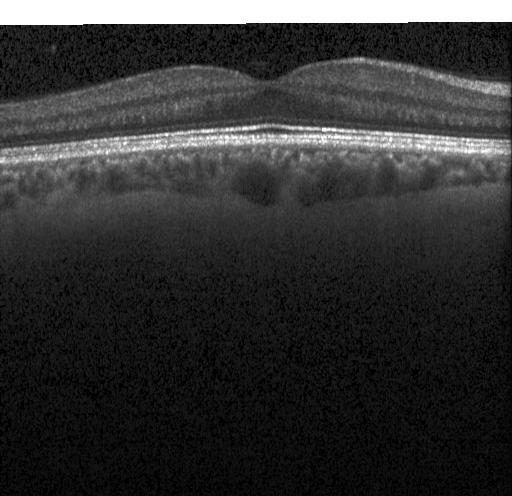

Instrument: Heidelberg Spectralis, spectral-domain optical coherence tomography, fovea-centered, optical coherence tomography scan.
The scan shows no choroidal neovascularization, no diabetic macular edema, and no drusen.